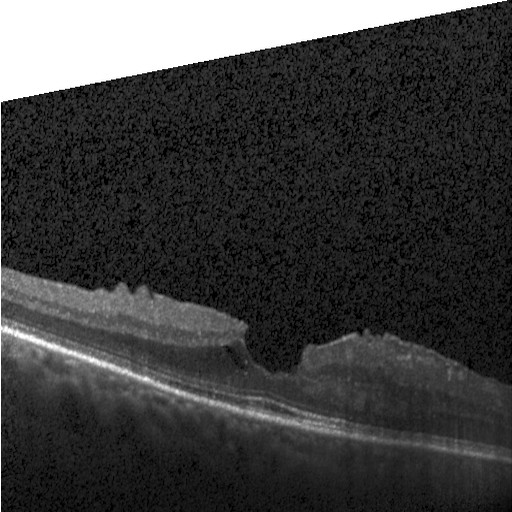 Diabetic macular edema (DME).